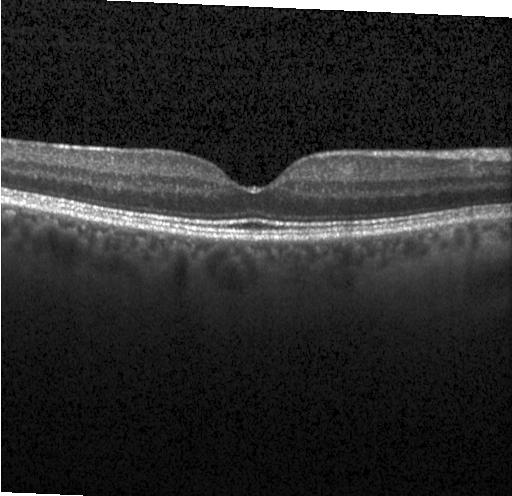 This B-scan demonstrates no choroidal neovascularization, no diabetic macular edema, and no drusen.